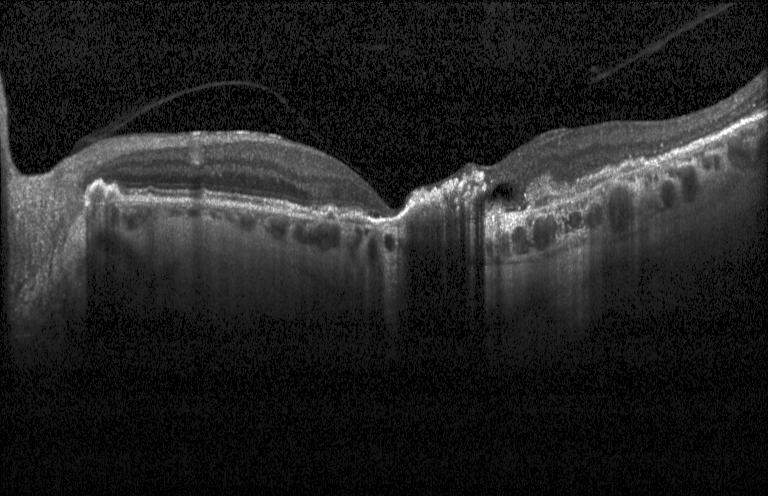

SD-OCT, centered on the fovea, Heidelberg Spectralis, retinal OCT cross-section
Diagnosis: a choroidal neovascular membrane.